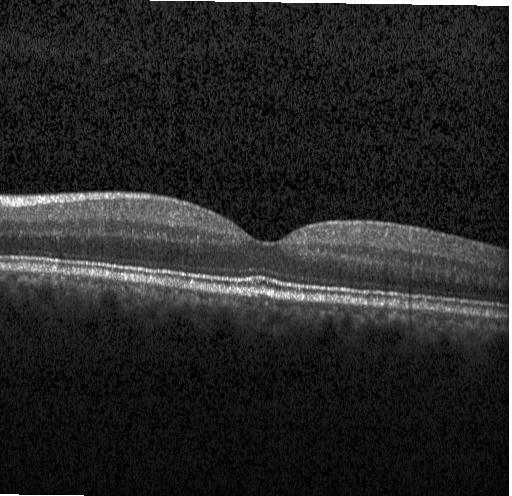 The scan shows no choroidal neovascularization, no diabetic macular edema, and no drusen.